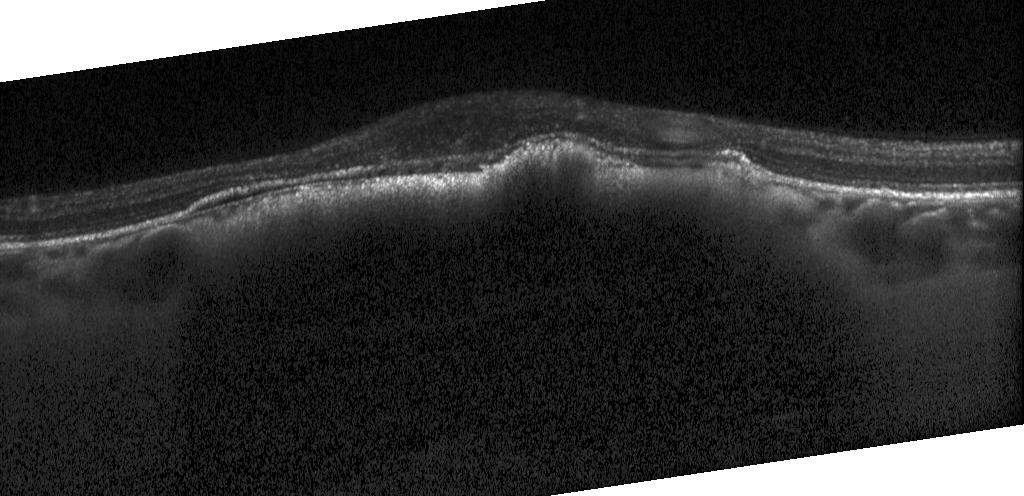 Spectral-domain OCT; optical coherence tomography scan; macular scan; Heidelberg Spectralis — Assessment: a choroidal neovascular membrane.